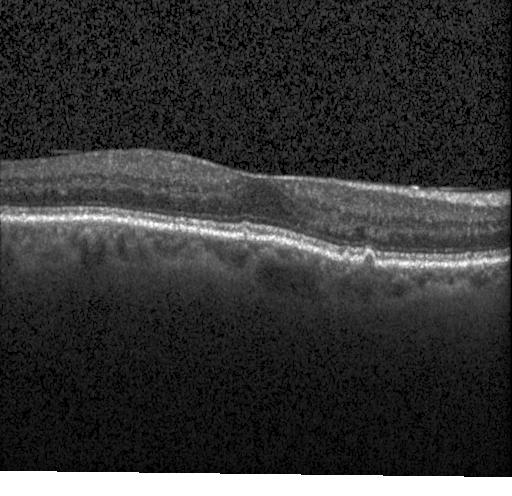 OCT B-scan, Heidelberg Spectralis OCT system, macular scan — The scan shows sub-RPE drusenoid deposits.